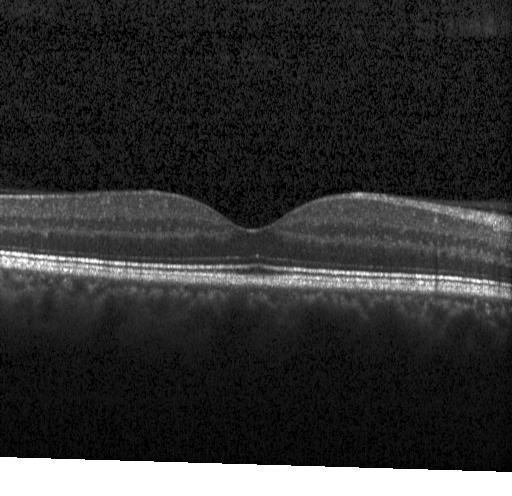

Acquired on a Heidelberg Spectralis, SD-OCT, OCT line scan.
Diagnosis: no evidence of CNV, DME, or drusen.